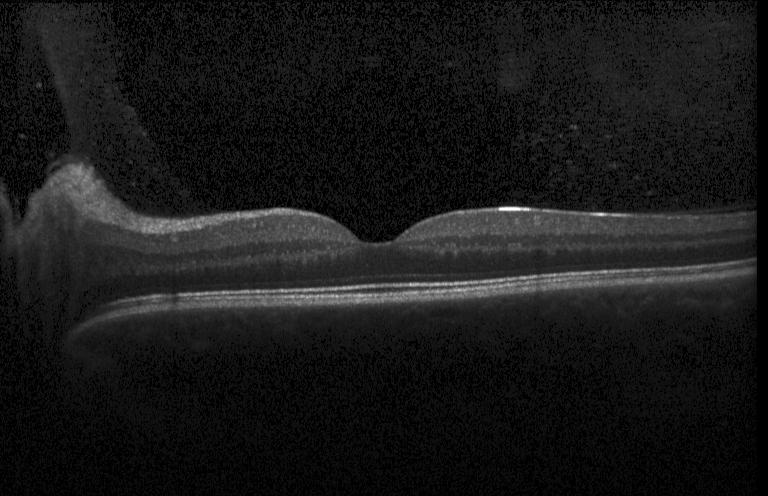 Finding: neither CNV, DME, nor drusen.